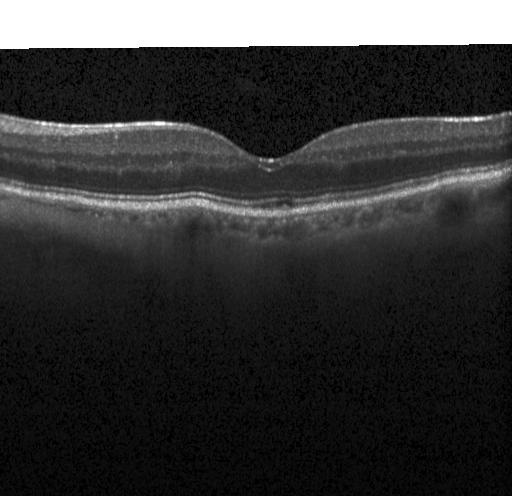 Optical coherence tomography scan; spectral-domain optical coherence tomography; fovea-centered; acquired on a Heidelberg Spectralis — Impression: neither choroidal neovascularization, diabetic macular edema, nor drusen.